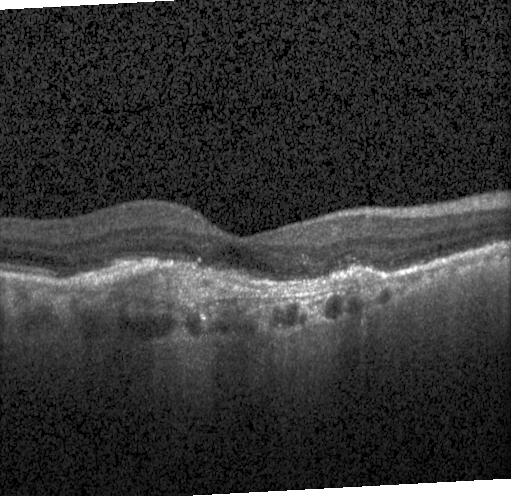

Horizontal scan through the fovea. Optical coherence tomography B-scan. Instrument: Heidelberg Spectralis. Spectral-domain OCT.
Impression: a choroidal neovascular membrane.